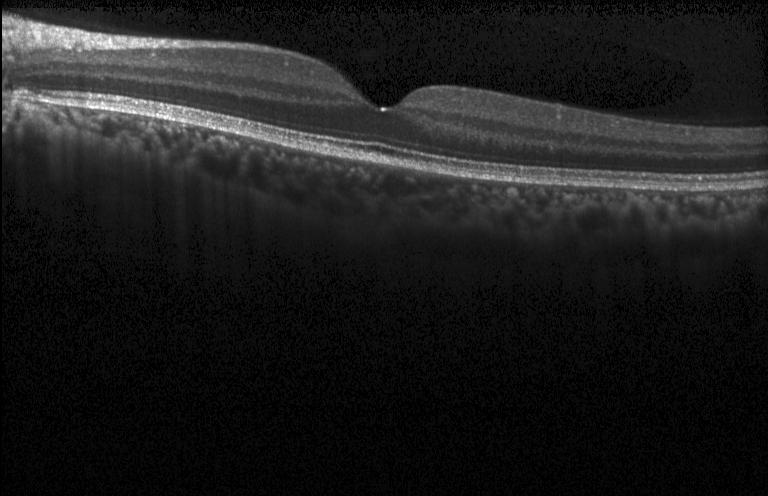
This B-scan demonstrates neither choroidal neovascularization, diabetic macular edema, nor drusen.